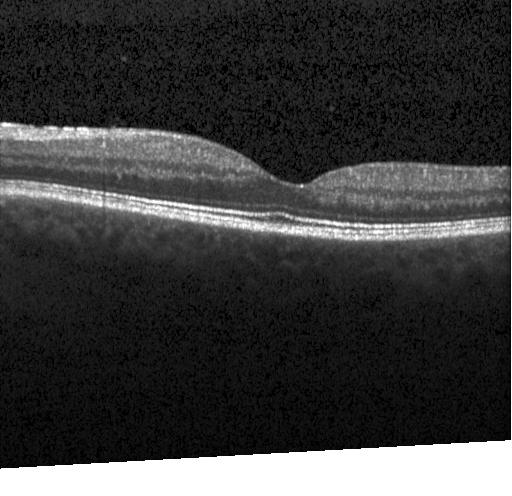 Retinal OCT B-scan. Impression: no evidence of choroidal neovascularization, diabetic macular edema, or drusen.